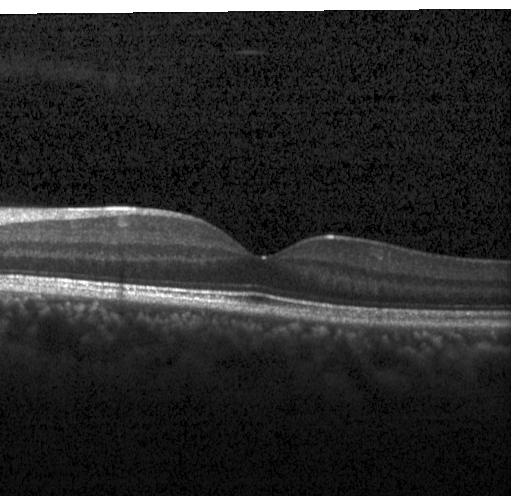
Finding: no evidence of choroidal neovascularization, diabetic macular edema, or drusen.